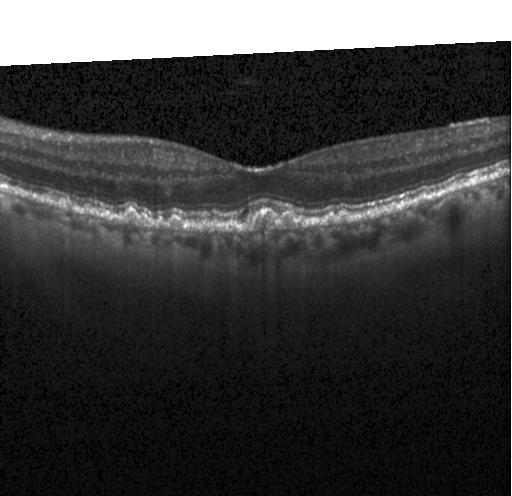 Macular OCT: sub-RPE drusenoid deposits.